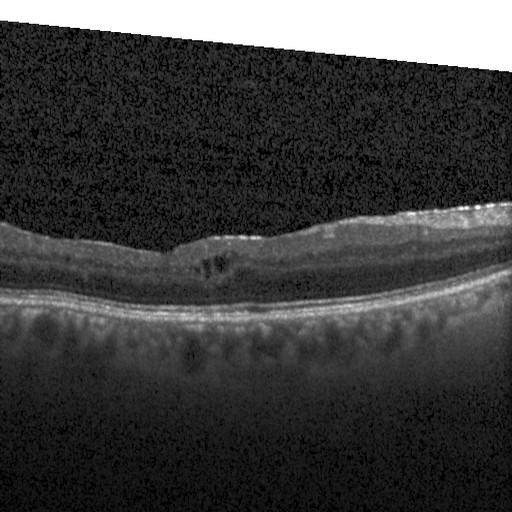 OCT line scan
Assessment: diabetic macular edema (DME).